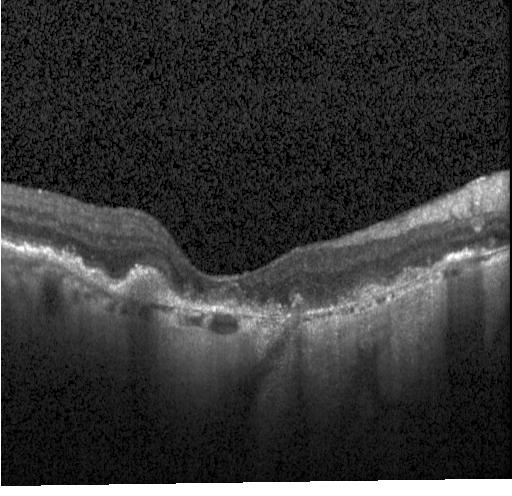
Assessment: CNV.